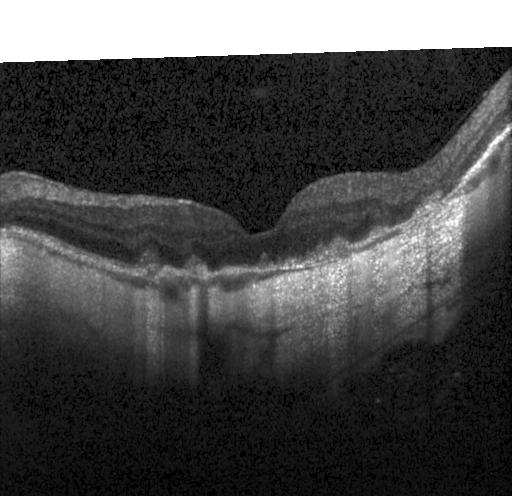
Horizontal scan through the fovea; retinal OCT B-scan; Heidelberg Spectralis
Finding: a choroidal neovascular membrane.